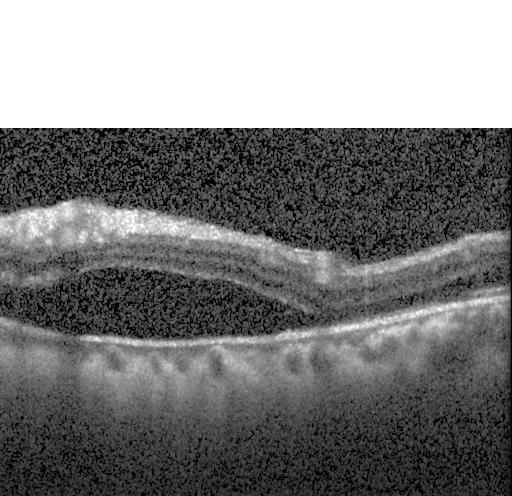 OCT B-scan · SD-OCT
The scan shows choroidal neovascularization (CNV).